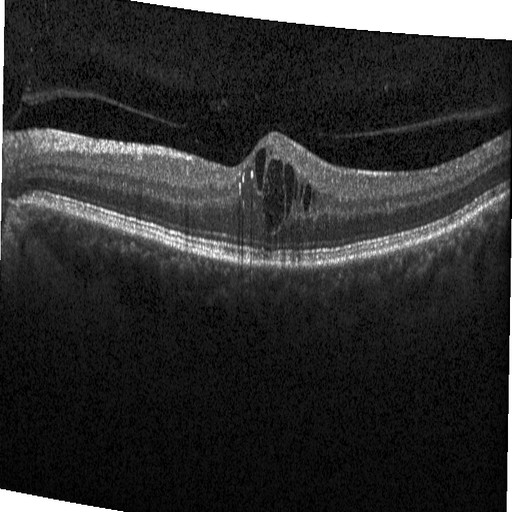 Retinal OCT cross-section showing diabetic macular edema (DME).